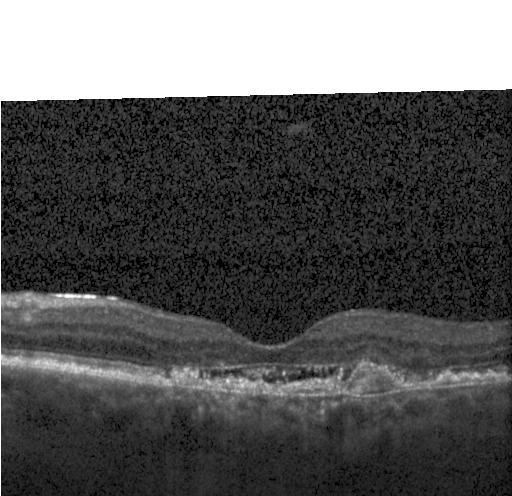
Through the macula, retinal OCT cross-section, Heidelberg Spectralis, spectral-domain optical coherence tomography
Macular OCT: CNV.